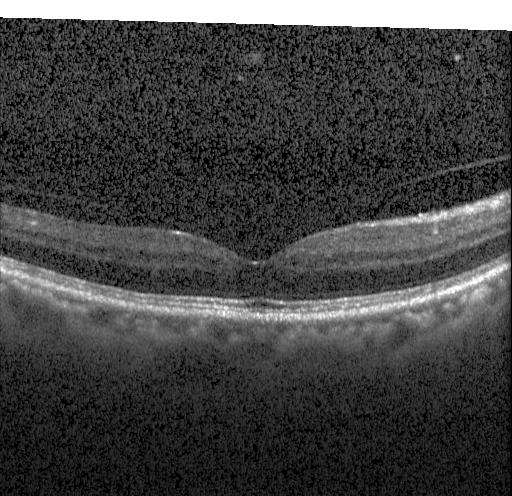
OCT scan showing no choroidal neovascularization, no diabetic macular edema, and no drusen.